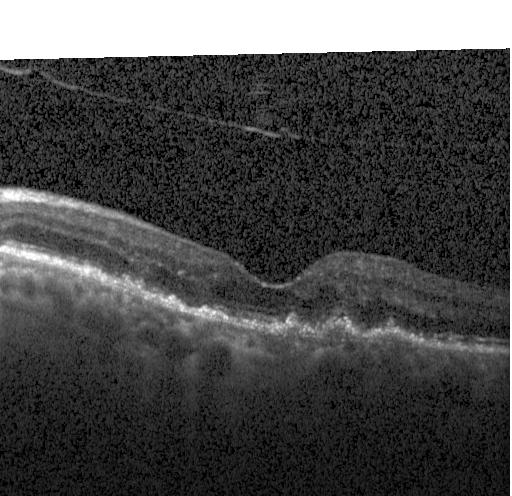
Horizontal scan through the fovea, optical coherence tomography scan — A choroidal neovascular membrane.